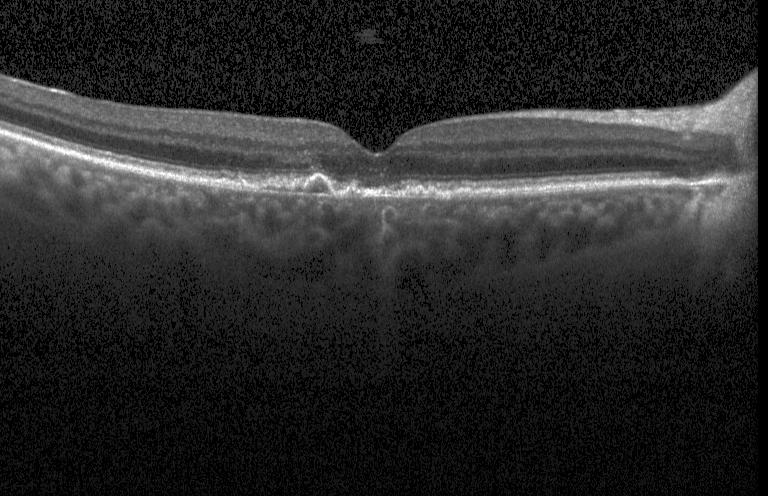 Macular OCT demonstrating a choroidal neovascular membrane.